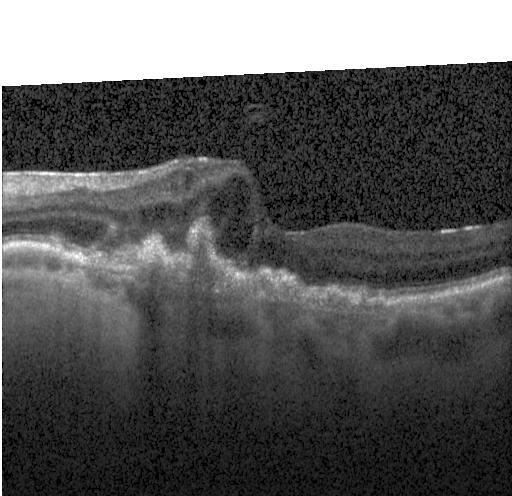

Acquired on a Heidelberg Spectralis, optical coherence tomography scan, horizontal scan through the fovea. Finding: a choroidal neovascular membrane.